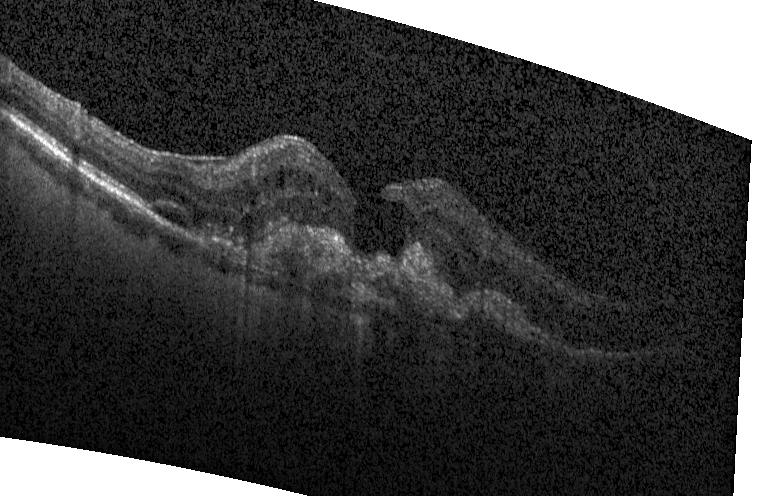

OCT B-scan — Impression: choroidal neovascularization.